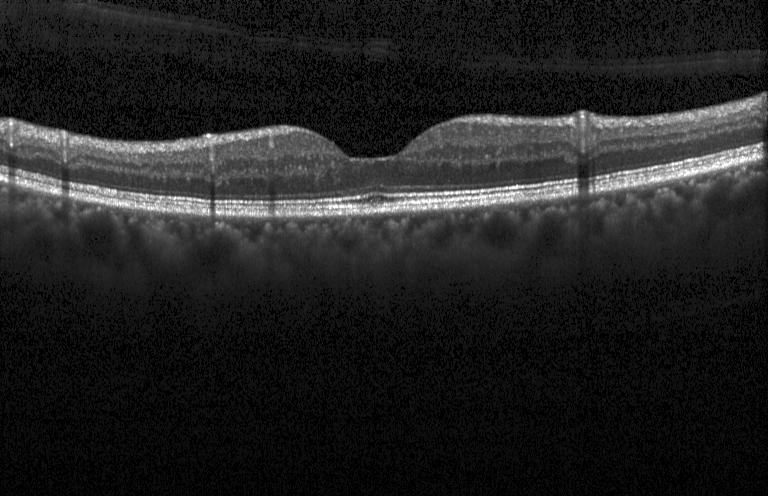

OCT finding: neither choroidal neovascularization, diabetic macular edema, nor drusen.